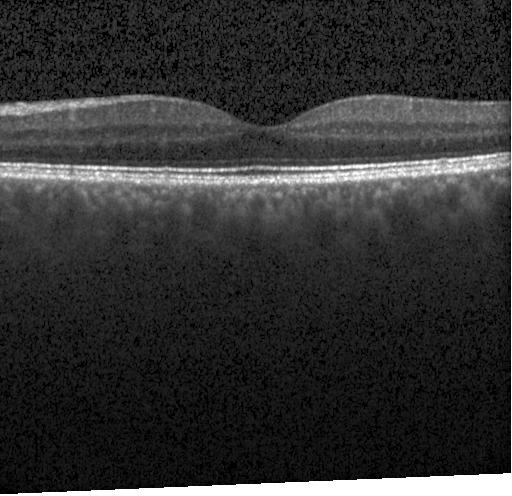
Macular OCT: neither choroidal neovascularization, diabetic macular edema, nor drusen.